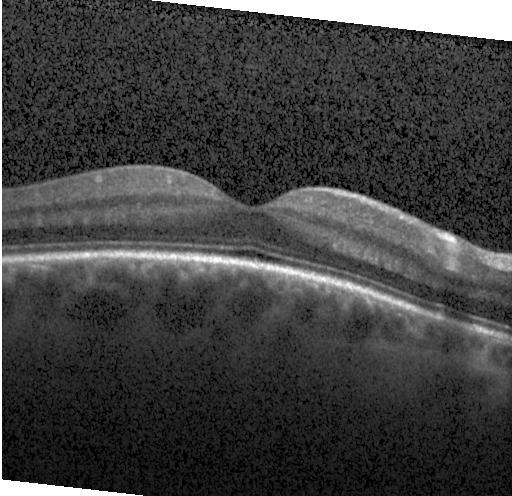

Assessment: neither choroidal neovascularization, diabetic macular edema, nor drusen.